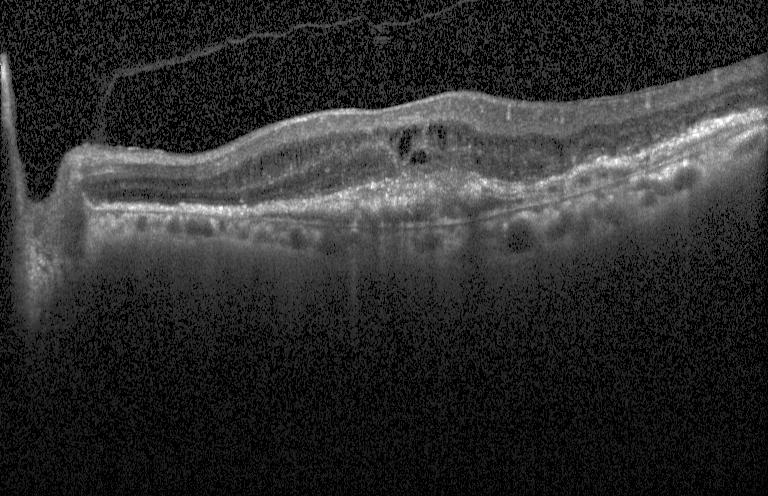

Retinal OCT B-scan.
Finding: a choroidal neovascular membrane.